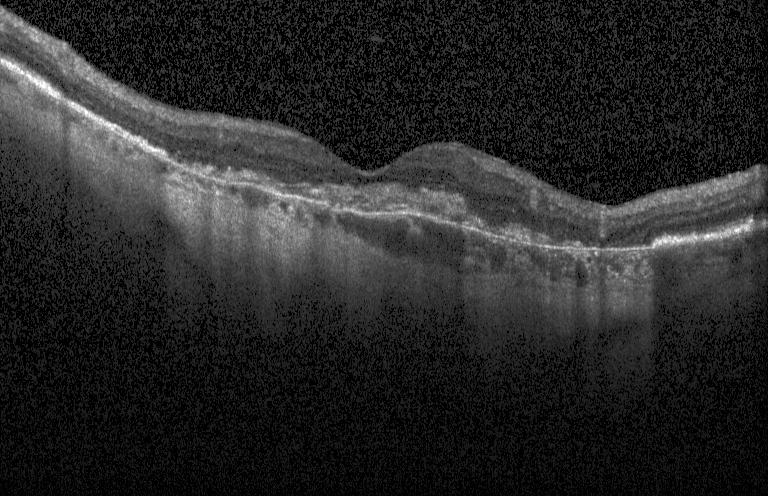 Macular OCT demonstrating CNV.